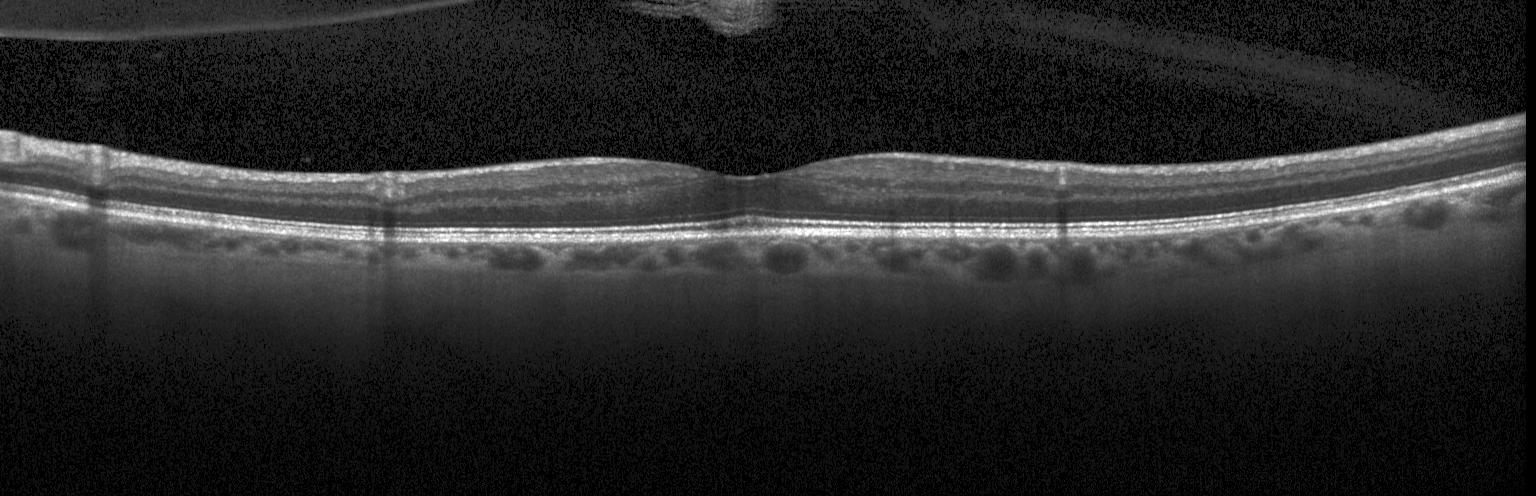 Retinal OCT cross-section.
Assessment: no CNV, no DME, and no drusen.